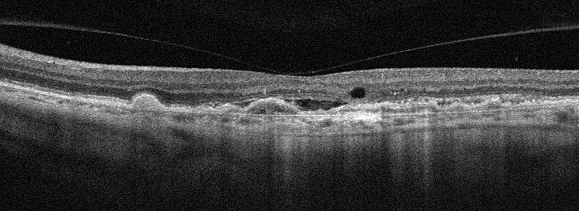

Oculus sinister, OCT B-scan, fovea-centered.
OCT finding: age-related macular degeneration (AMD).